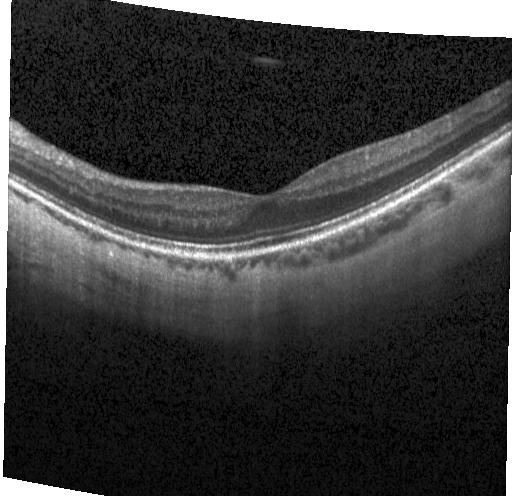
Retinal OCT B-scan, acquired on a Heidelberg Spectralis, spectral-domain OCT, horizontal scan through the fovea
Impression: no evidence of CNV, DME, or drusen.